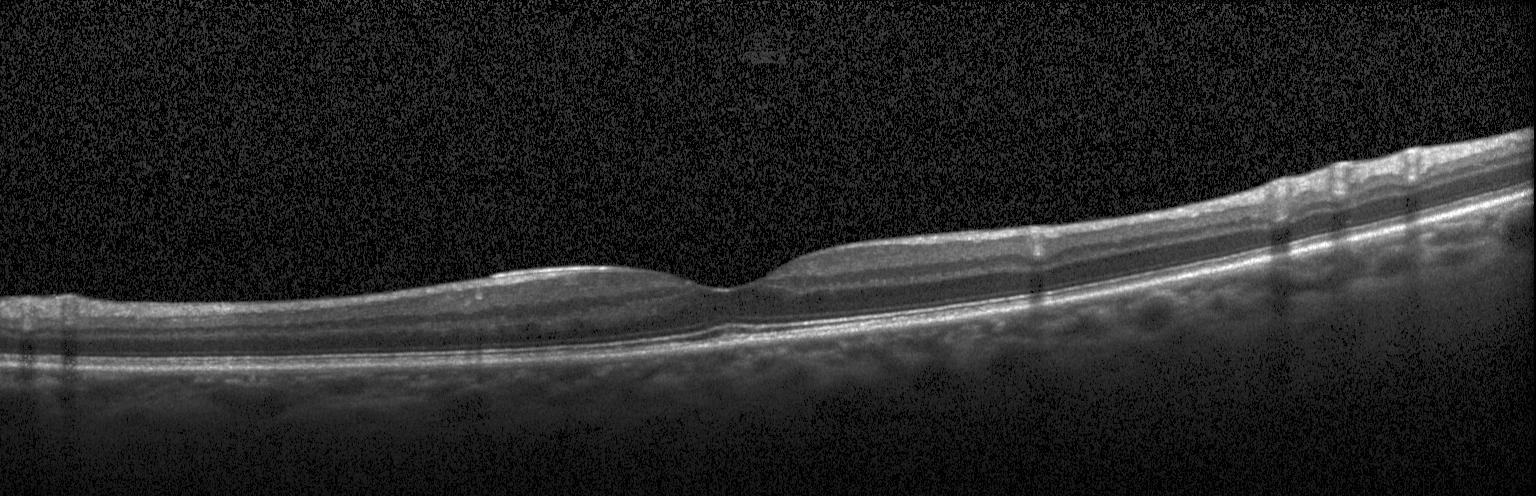
Retinal OCT cross-section
No choroidal neovascularization, diabetic macular edema, or drusen.